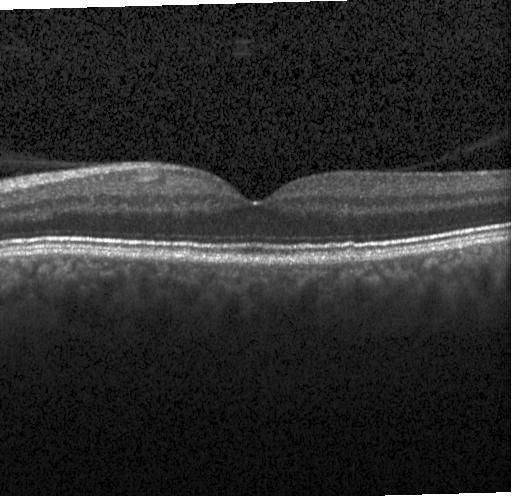
Finding: neither choroidal neovascularization, diabetic macular edema, nor drusen.